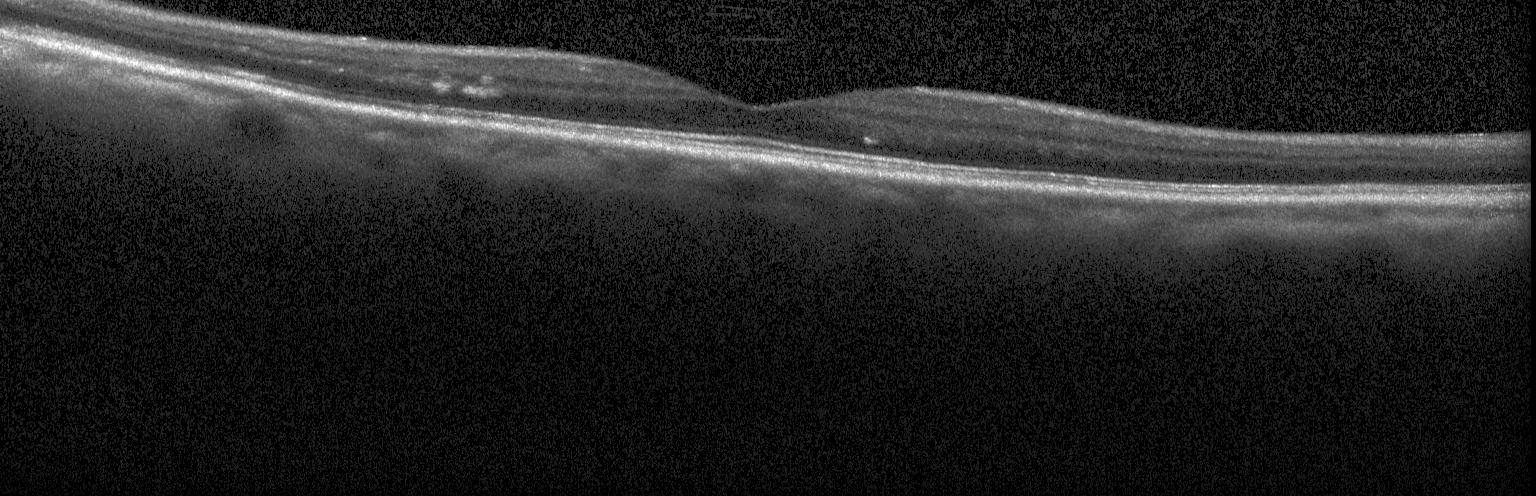
Finding: no evidence of choroidal neovascularization, diabetic macular edema, or drusen.